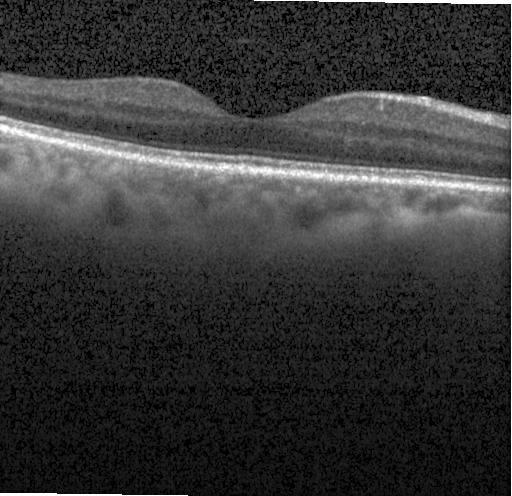

Through the macula, spectral-domain optical coherence tomography, OCT line scan, Heidelberg Spectralis OCT system
Impression: neither choroidal neovascularization, diabetic macular edema, nor drusen.